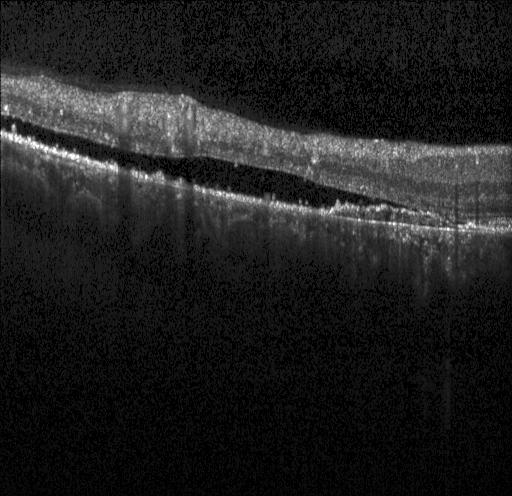 Spectral-domain OCT; retinal OCT B-scan. Finding: a choroidal neovascular membrane.